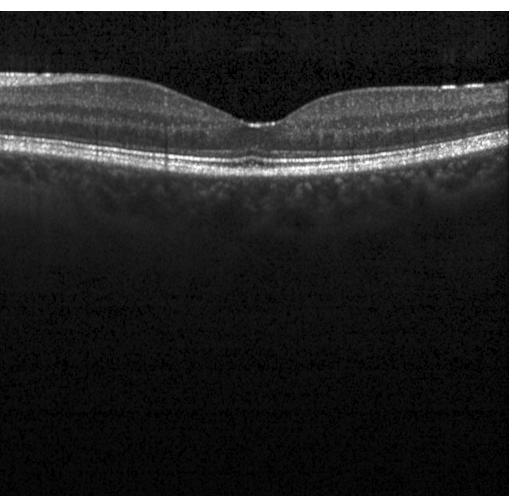

This B-scan demonstrates neither choroidal neovascularization, diabetic macular edema, nor drusen.